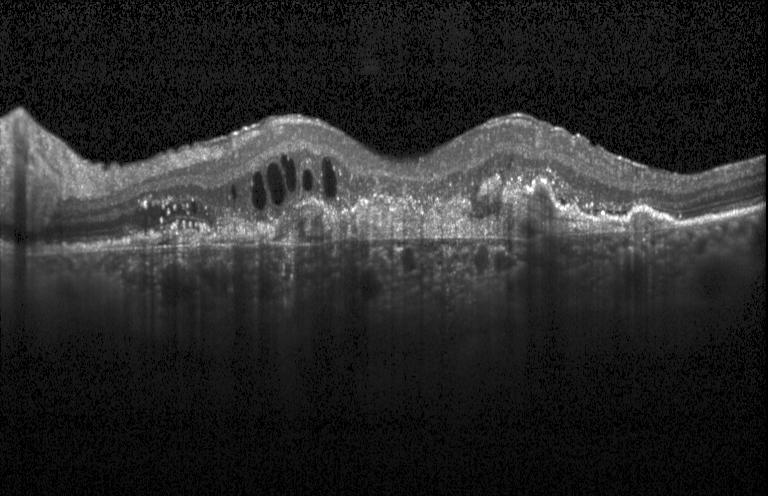
Impression: choroidal neovascularization (CNV).